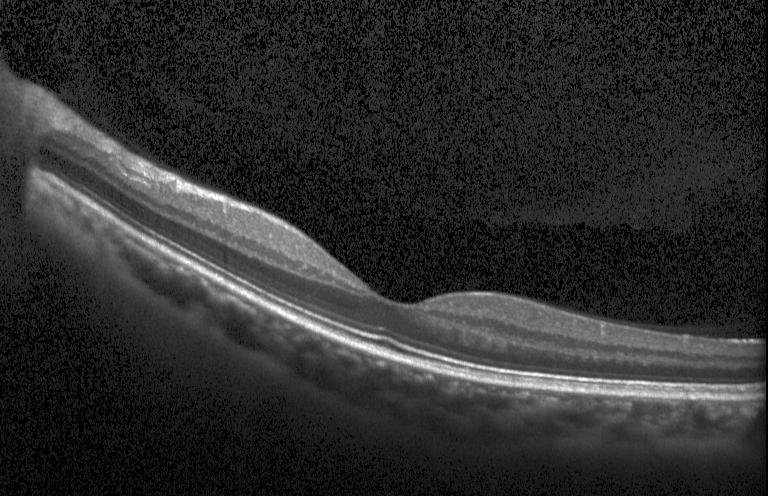

Assessment: no choroidal neovascularization, no diabetic macular edema, and no drusen.